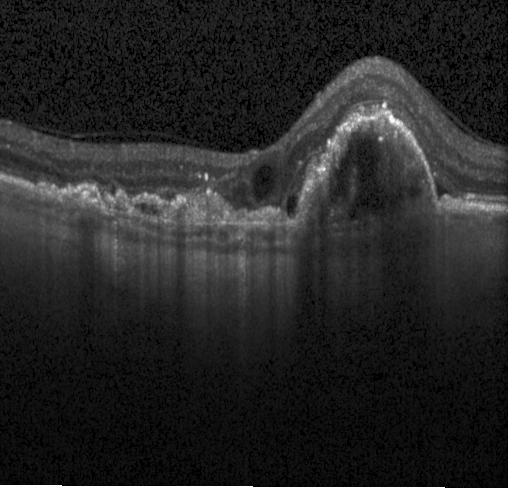 Optical coherence tomography scan, instrument: Heidelberg Spectralis, centered on the fovea.
Finding: a choroidal neovascular membrane.